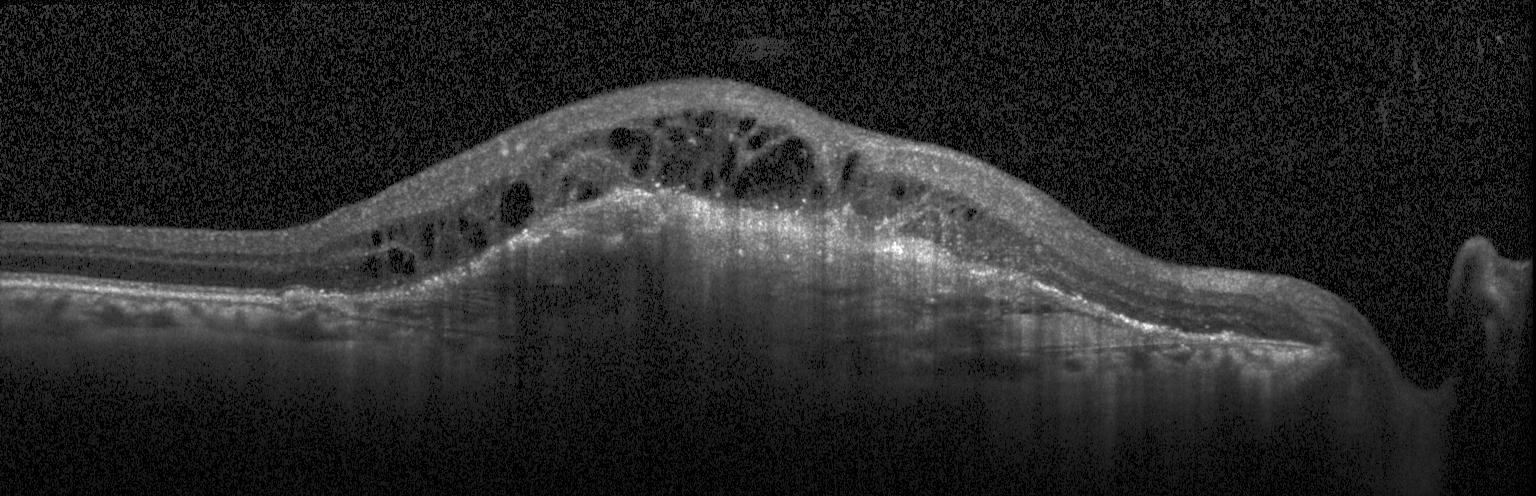

Optical coherence tomography scan. Acquired on a Heidelberg Spectralis — OCT finding: a choroidal neovascular membrane.